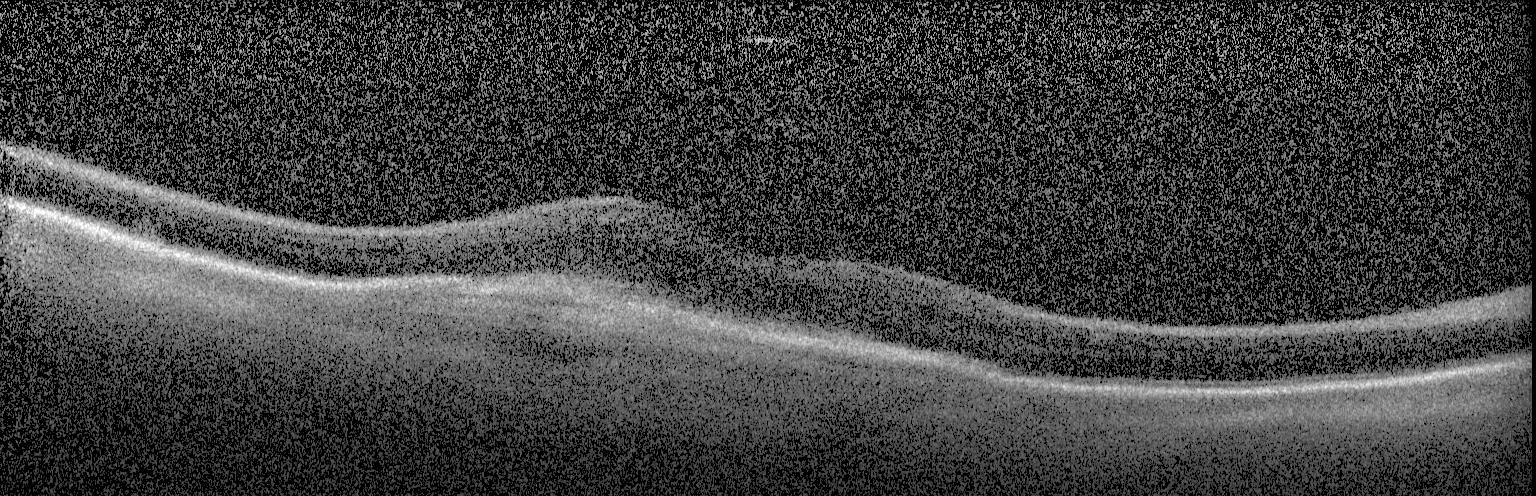

OCT B-scan, spectral-domain optical coherence tomography, instrument: Heidelberg Spectralis — Diagnosis: a choroidal neovascular membrane.